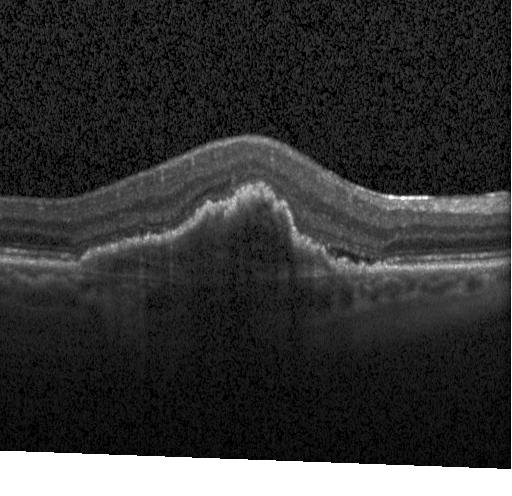

This B-scan demonstrates a choroidal neovascular membrane.